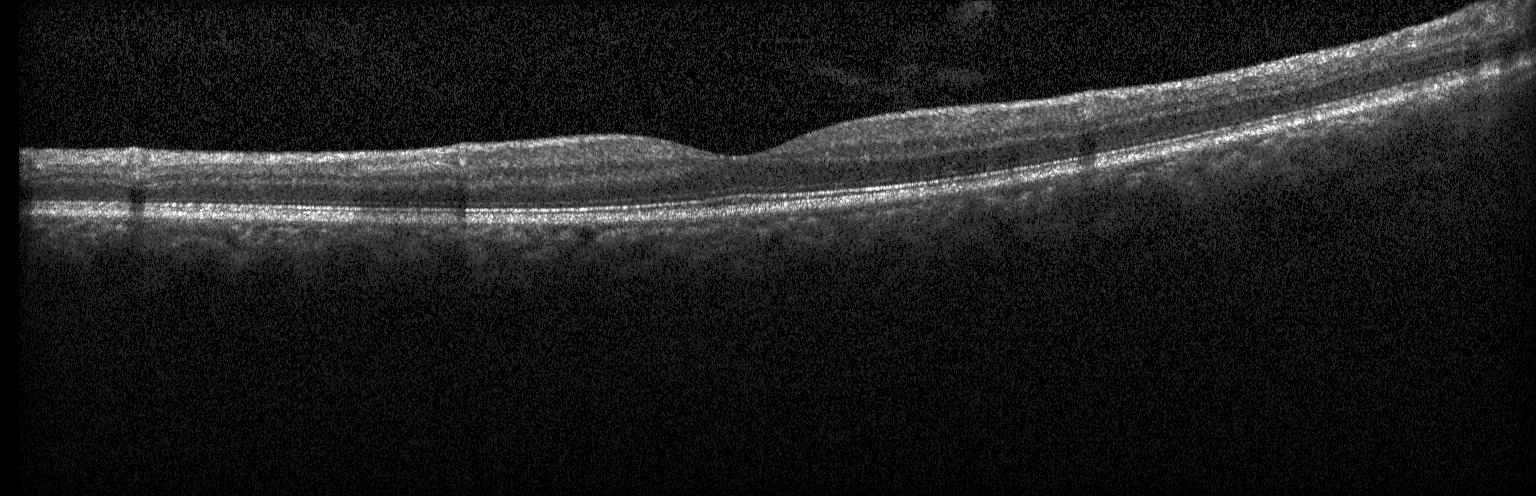
Spectral-domain OCT, centered on the fovea, acquired on a Heidelberg Spectralis, retinal OCT cross-section. This B-scan demonstrates no CNV, DME, or drusen.